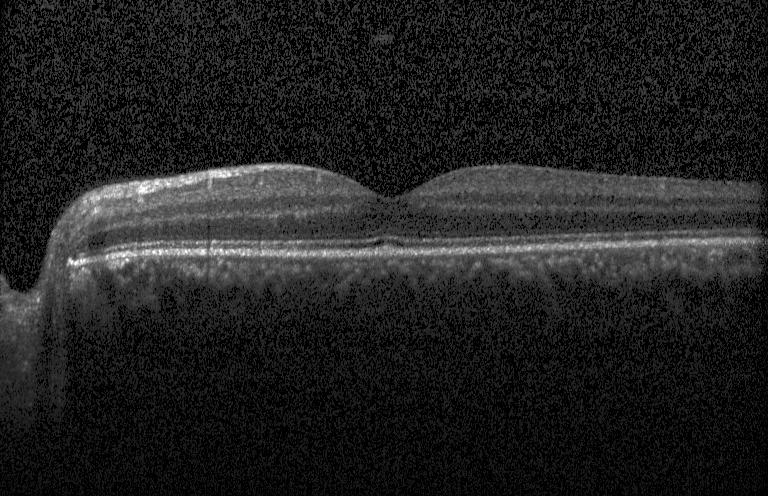 Optical coherence tomography B-scan, instrument: Heidelberg Spectralis, horizontal scan through the fovea.
Impression: no CNV, no DME, and no drusen.